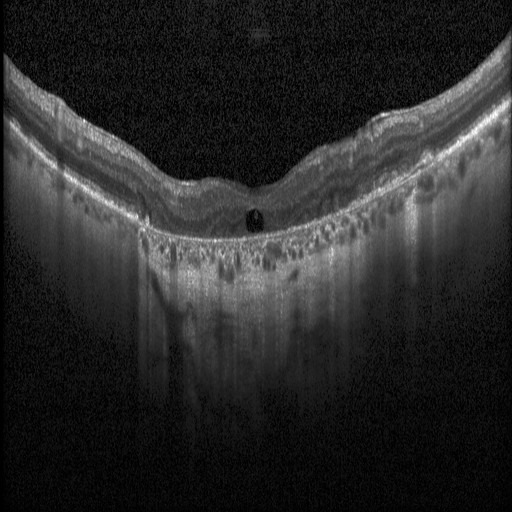
Dx: diabetic macular edema.